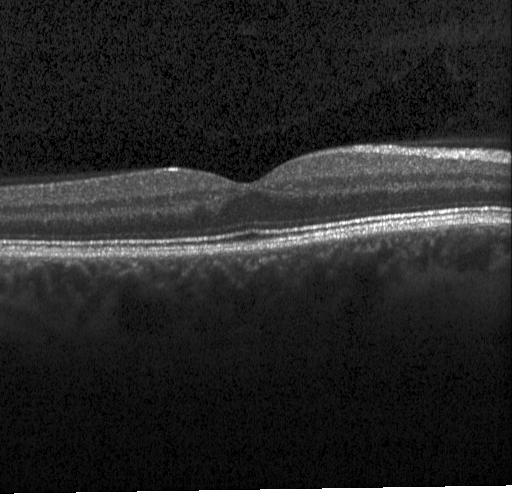
OCT B-scan
Assessment: neither choroidal neovascularization, diabetic macular edema, nor drusen.